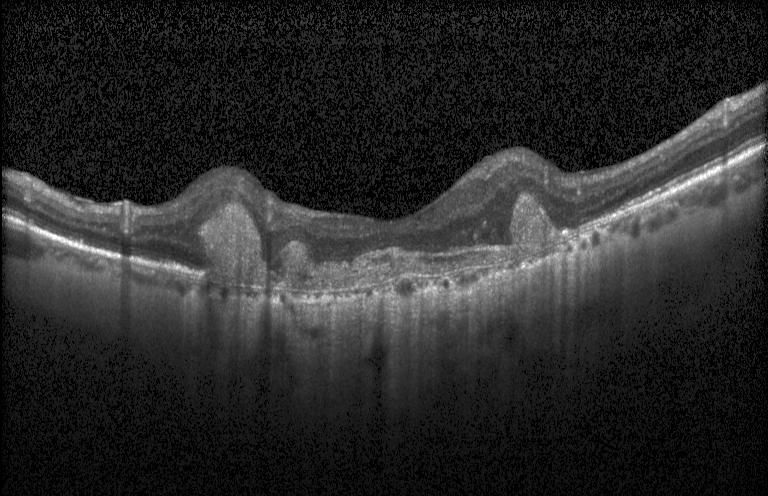
Retinal OCT cross-section. The scan shows CNV.